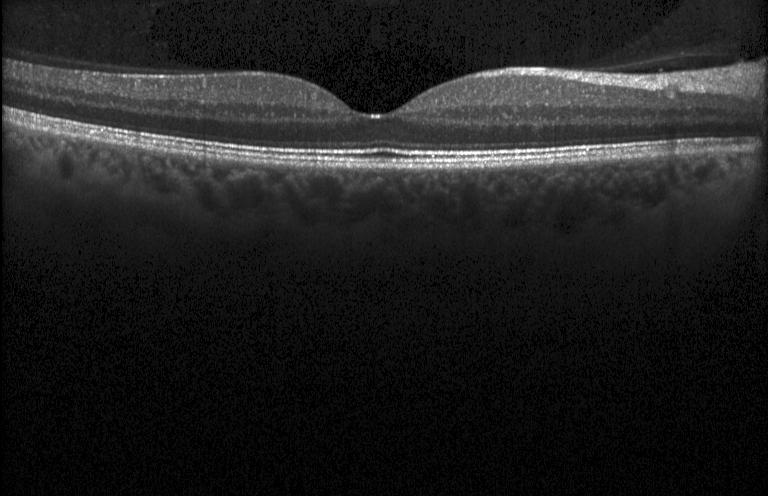

OCT B-scan showing no CNV, DME, or drusen.